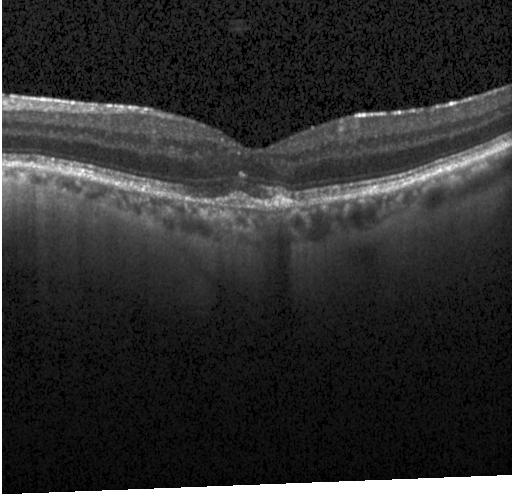
Macular OCT demonstrating CNV.